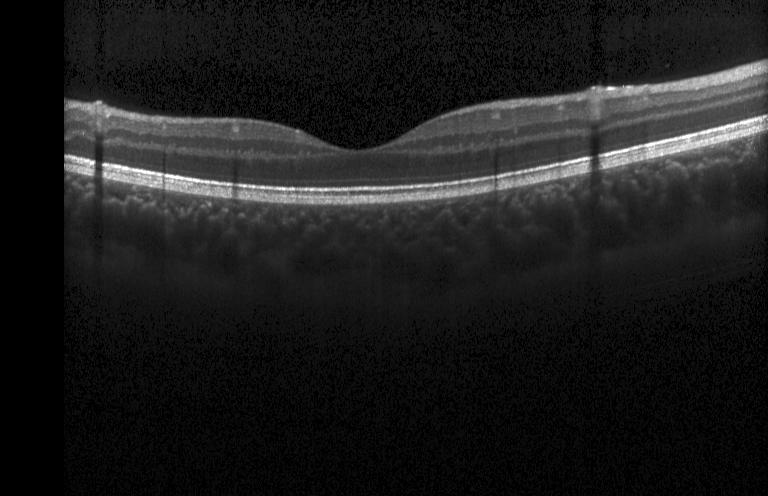

OCT finding: no evidence of CNV, DME, or drusen.